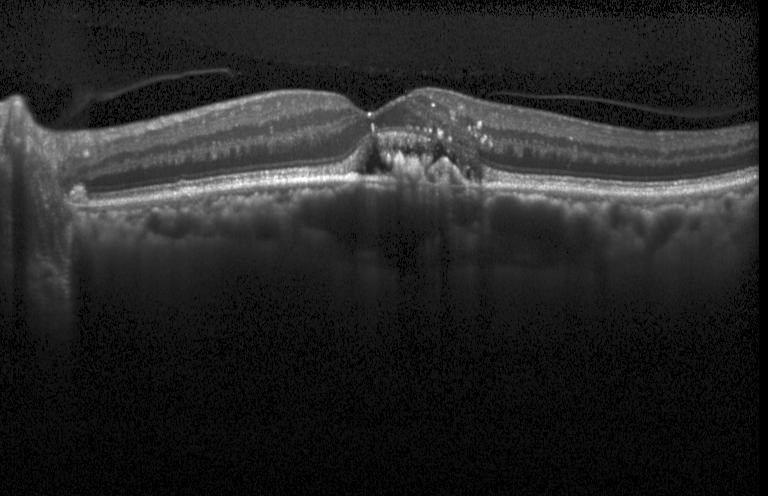 Heidelberg Spectralis; retinal OCT cross-section; spectral-domain optical coherence tomography; fovea-centered. Assessment: CNV.